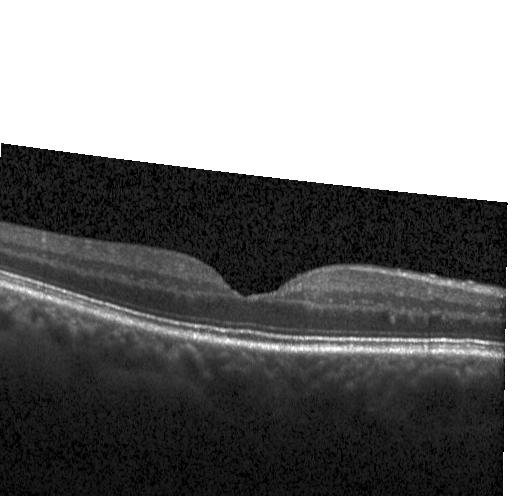 Heidelberg Spectralis. OCT B-scan
The scan shows neither choroidal neovascularization, diabetic macular edema, nor drusen.